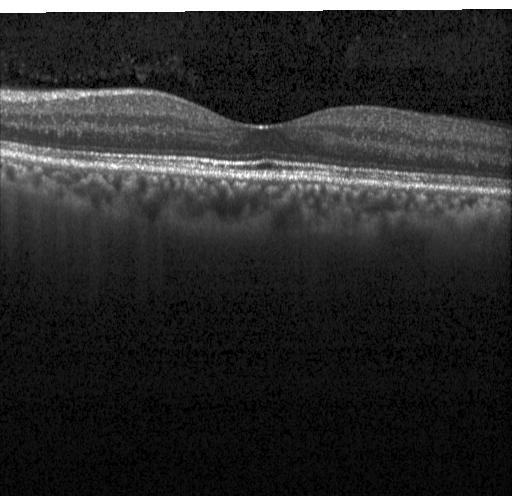 OCT B-scan showing no evidence of choroidal neovascularization, diabetic macular edema, or drusen.